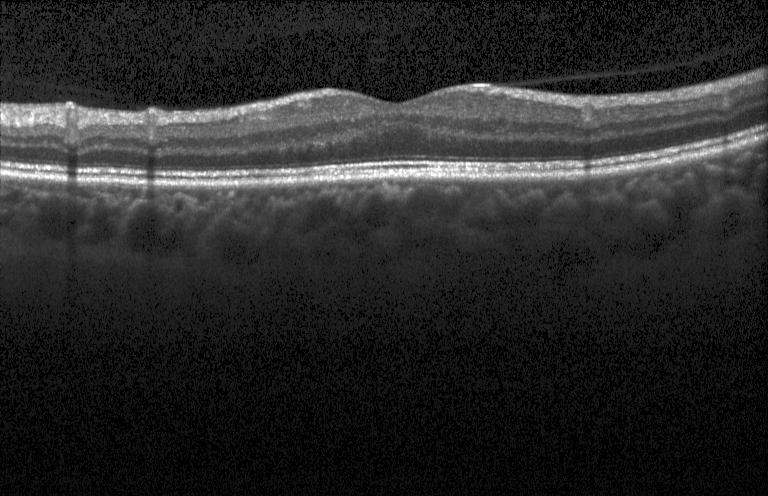
Diagnosis: neither CNV, DME, nor drusen.